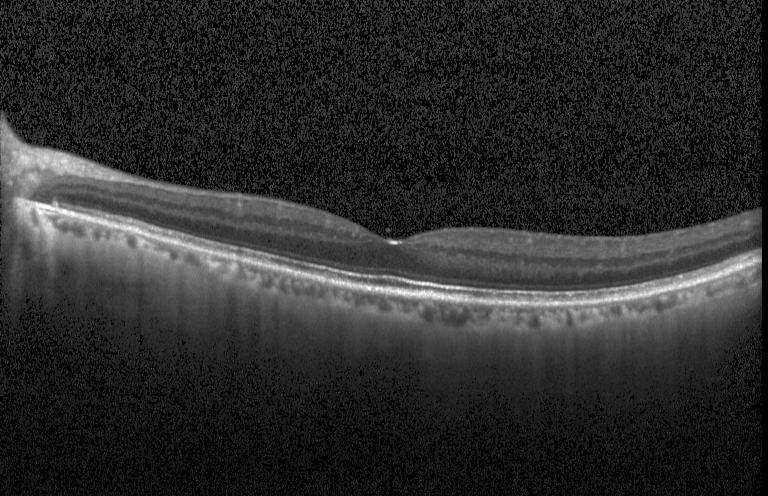 Retinal OCT cross-section. Impression: no choroidal neovascularization, no diabetic macular edema, and no drusen.